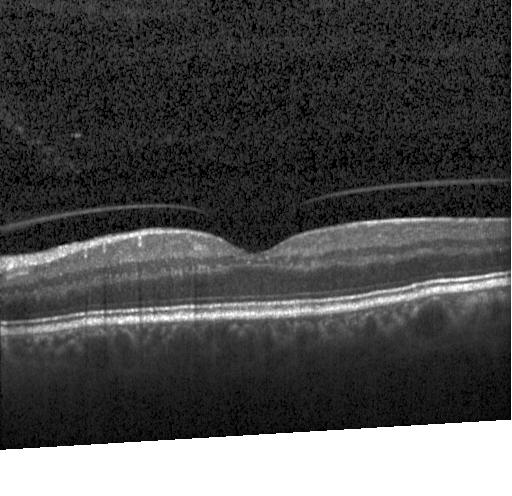

Retinal OCT B-scan. Impression: no choroidal neovascularization, diabetic macular edema, or drusen.